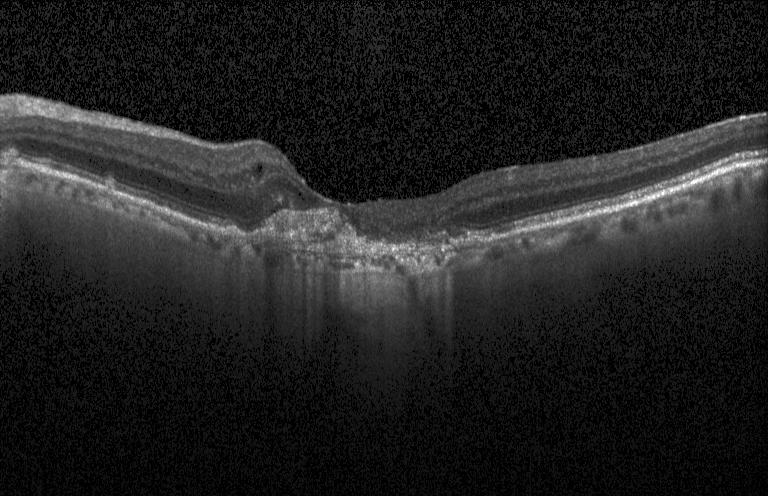
Heidelberg Spectralis OCT system. Optical coherence tomography scan. Spectral-domain OCT. Through the macula — Assessment: choroidal neovascularization.